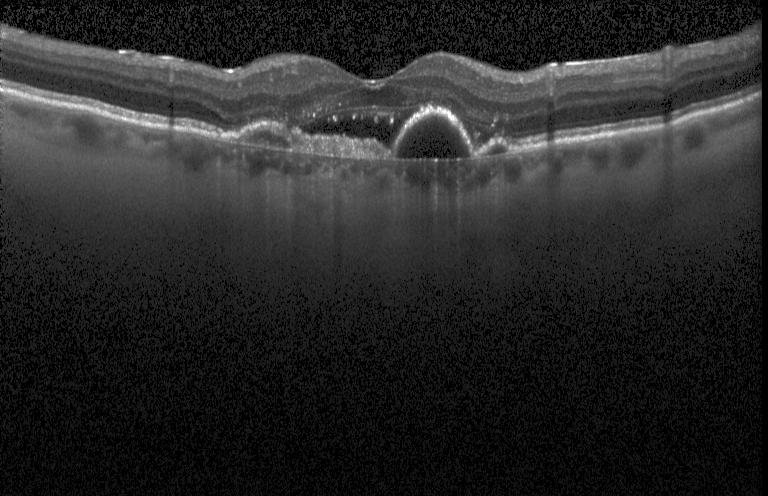

Heidelberg Spectralis; spectral-domain optical coherence tomography; through the macula; retinal OCT B-scan
Choroidal neovascularization (CNV).